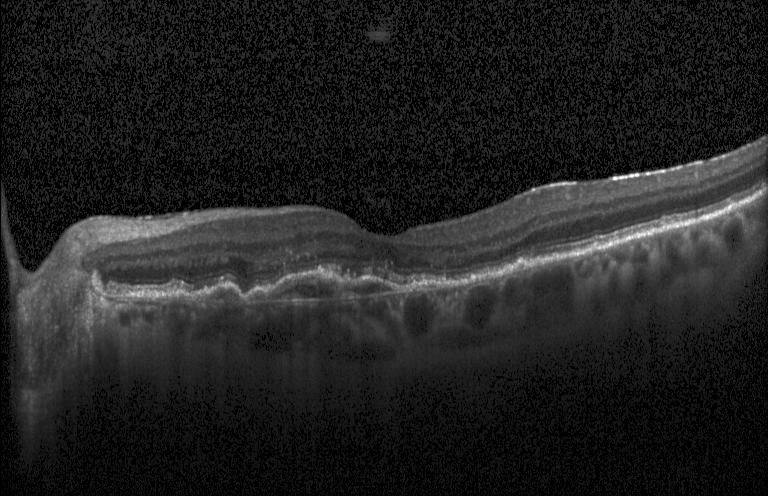
Retinal OCT cross-section — Assessment: a choroidal neovascular membrane.